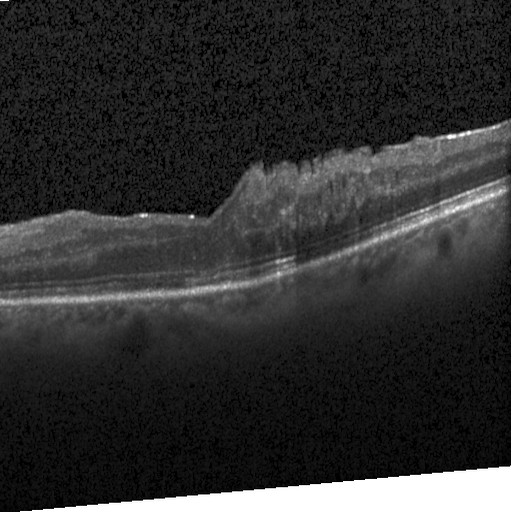
Diagnosis: diabetic macular edema.